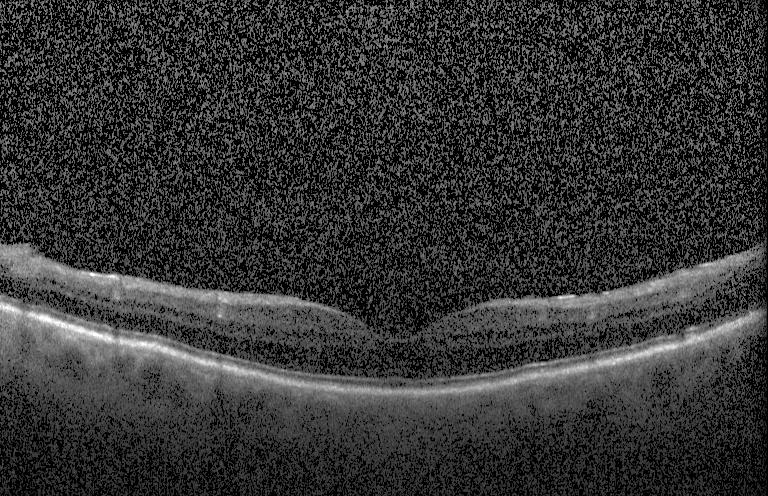 Diagnosis: neither choroidal neovascularization, diabetic macular edema, nor drusen.